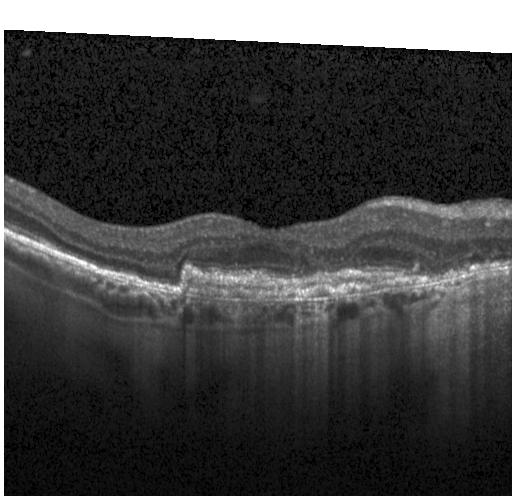

Instrument: Heidelberg Spectralis, retinal OCT B-scan, centered on the fovea, SD-OCT. Impression: CNV.